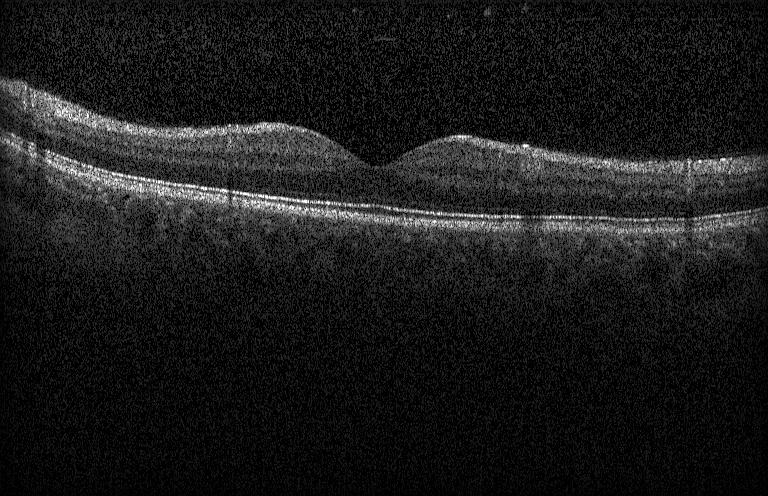

Diagnosis: no choroidal neovascularization, diabetic macular edema, or drusen.